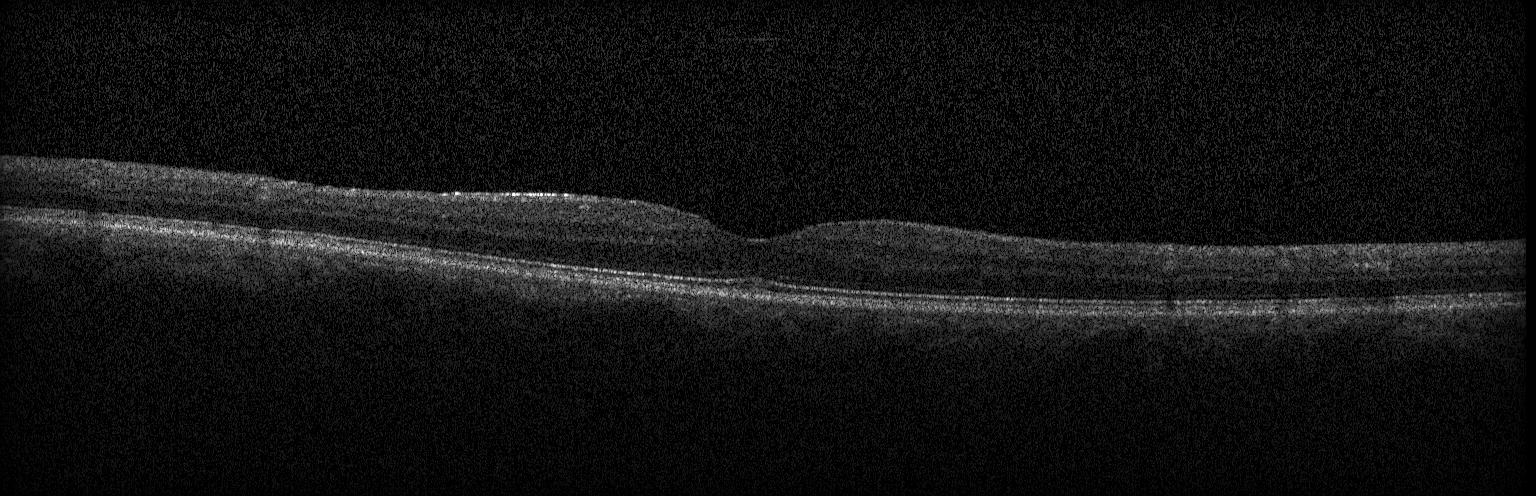

Heidelberg Spectralis; retinal OCT cross-section — Impression: no evidence of choroidal neovascularization, diabetic macular edema, or drusen.